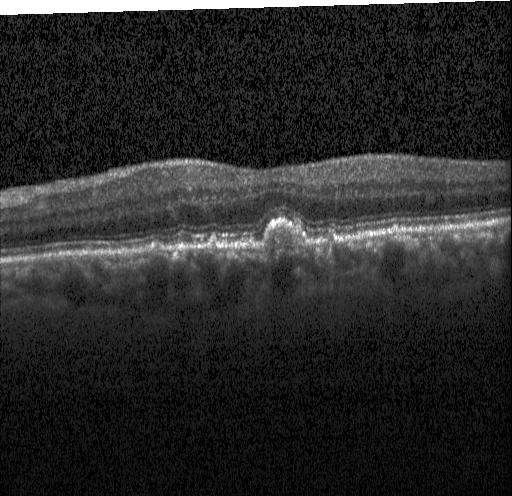
Spectral-domain optical coherence tomography; centered on the fovea; retinal OCT B-scan; Heidelberg Spectralis OCT system. Multiple drusen.